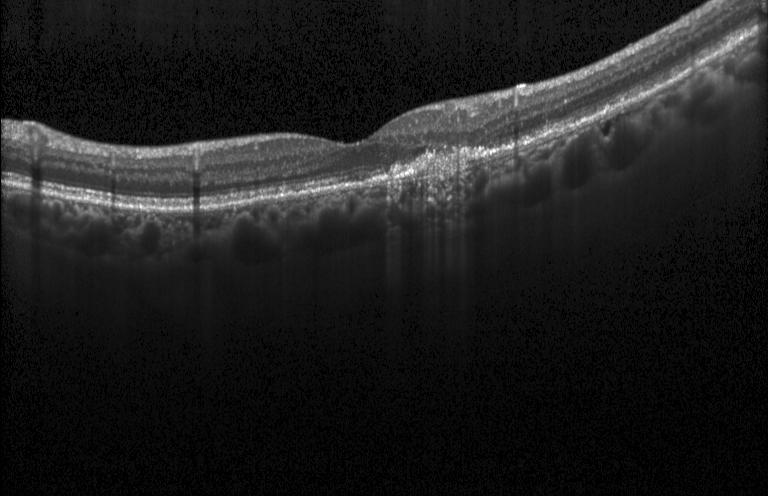 Optical coherence tomography B-scan · Heidelberg Spectralis OCT system. Choroidal neovascularization (CNV).